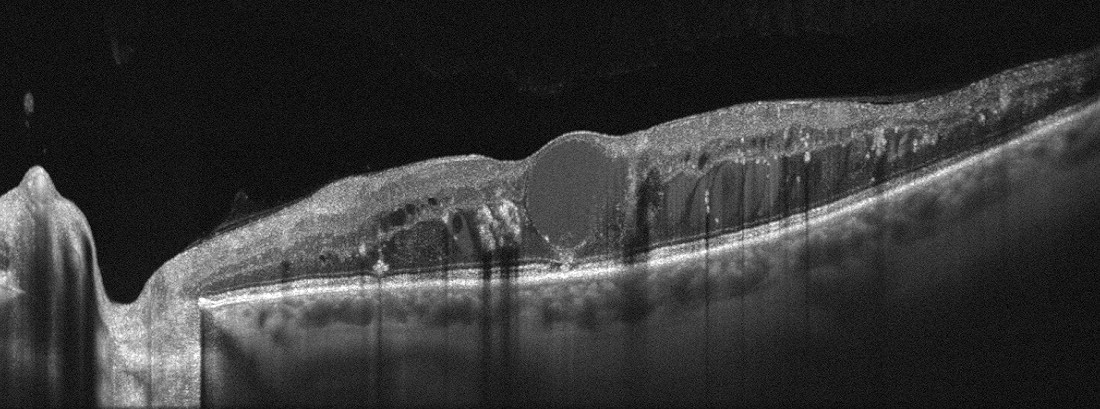

Diagnosis: DME.